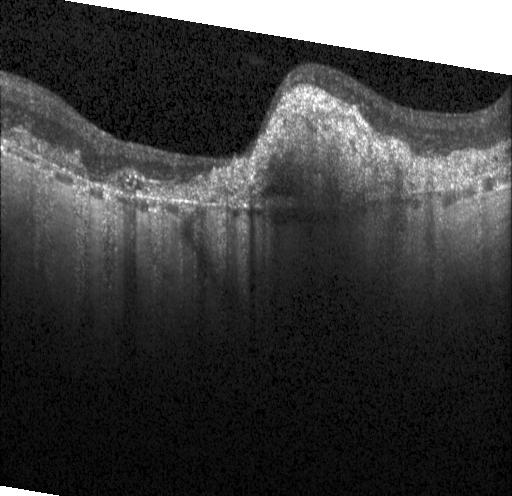 OCT B-scan — Macular OCT: a choroidal neovascular membrane.